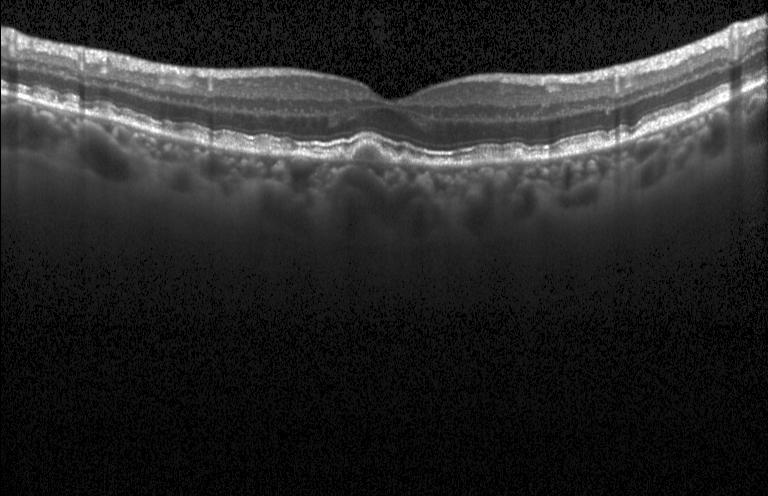

Retinal OCT B-scan — Assessment: multiple drusen.